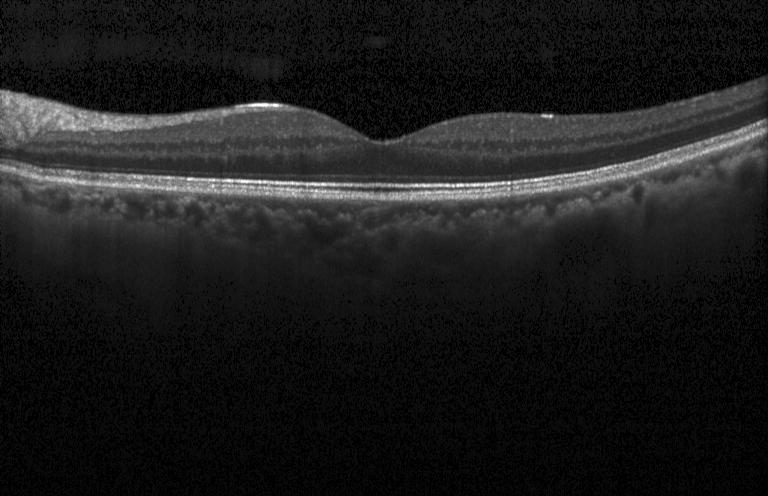

No choroidal neovascularization, diabetic macular edema, or drusen.